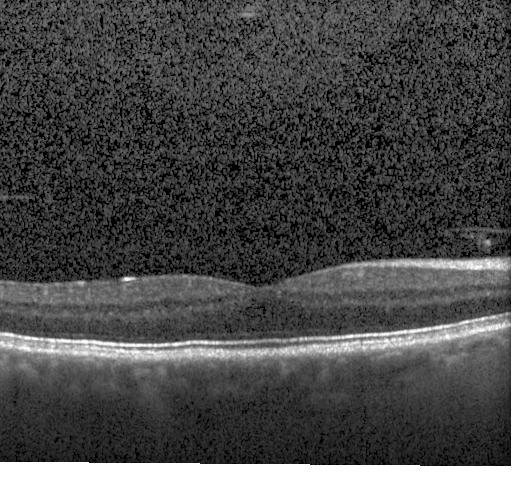

Finding: no choroidal neovascularization, no diabetic macular edema, and no drusen.